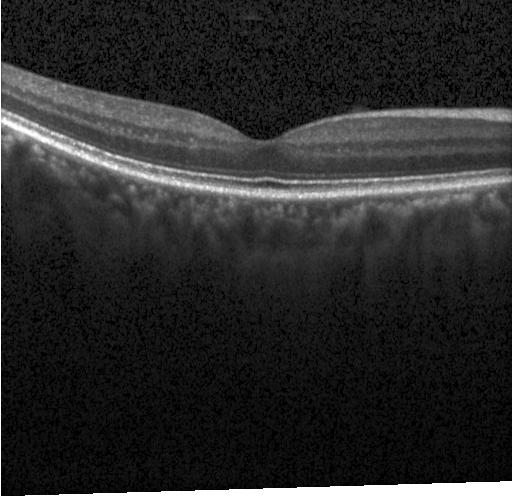

Macular OCT demonstrating no choroidal neovascularization, no diabetic macular edema, and no drusen.